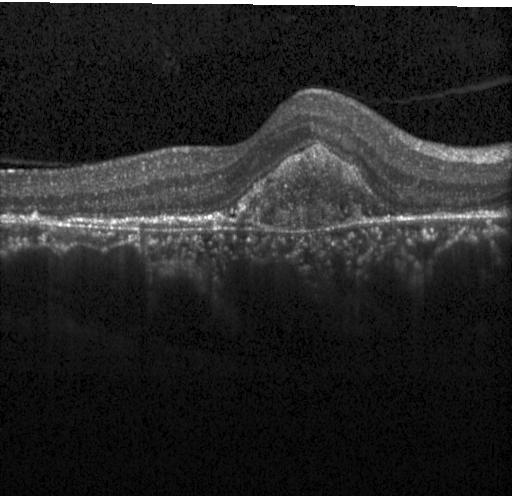
OCT B-scan
Dx: choroidal neovascularization.